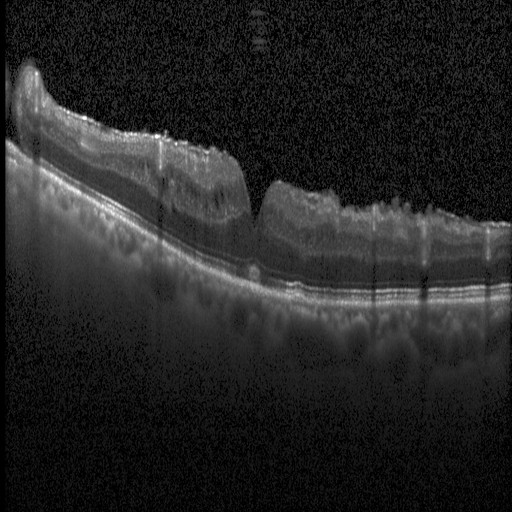
Spectral-domain optical coherence tomography, retinal OCT cross-section, Heidelberg Spectralis OCT system
Impression: DME.